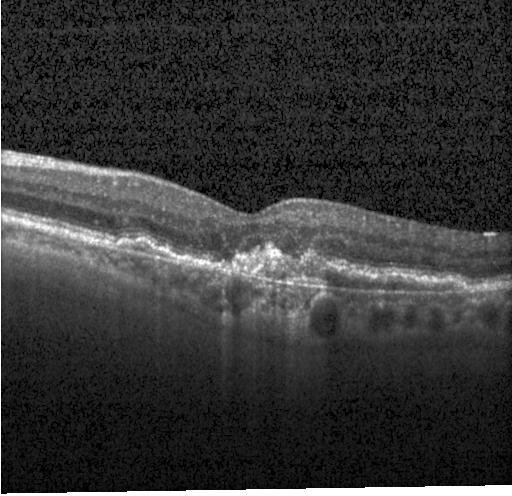

Spectral-domain OCT B-scan: a choroidal neovascular membrane.